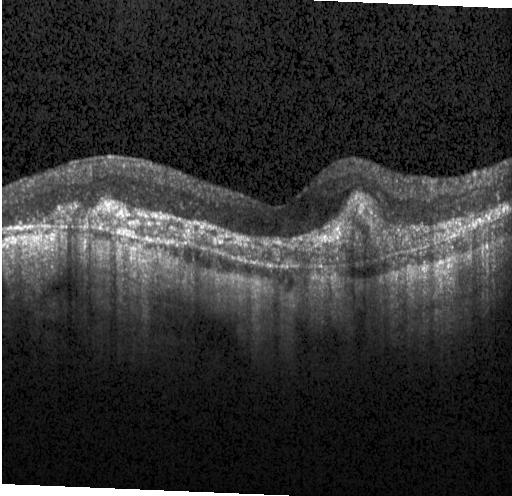 Retinal OCT B-scan.
Diagnosis: a choroidal neovascular membrane.